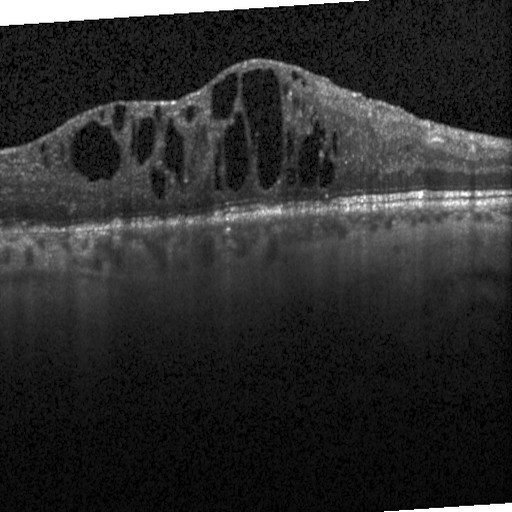 OCT finding: diabetic macular edema.